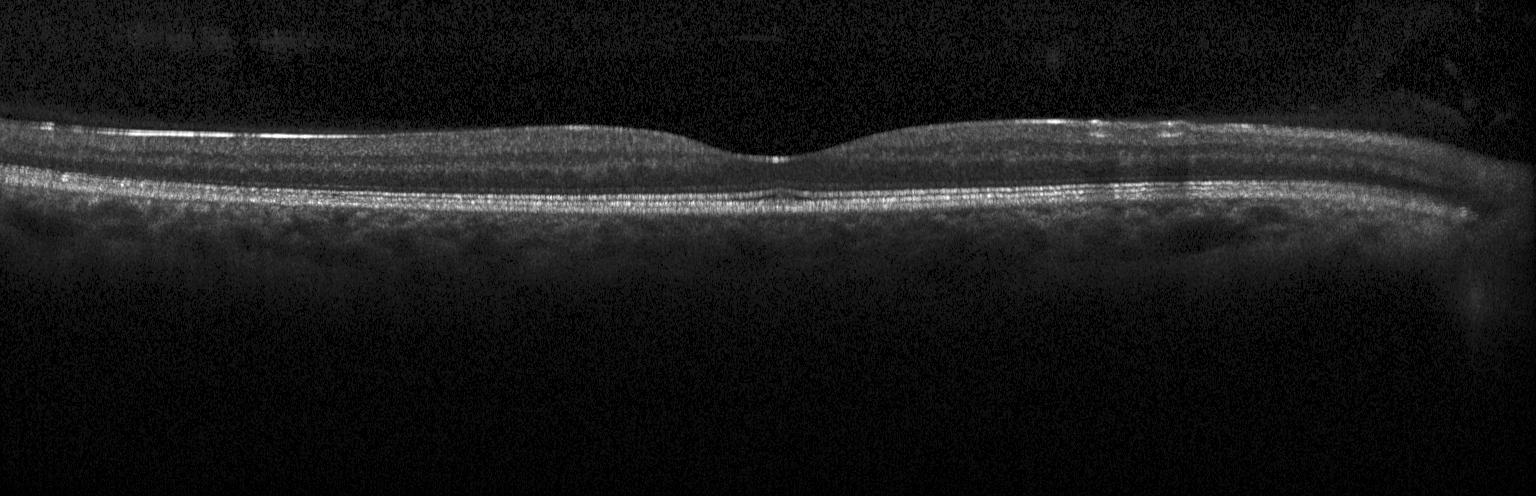
Centered on the fovea. Acquired on a Heidelberg Spectralis. Spectral-domain OCT. Retinal OCT cross-section.
Finding: no choroidal neovascularization, no diabetic macular edema, and no drusen.